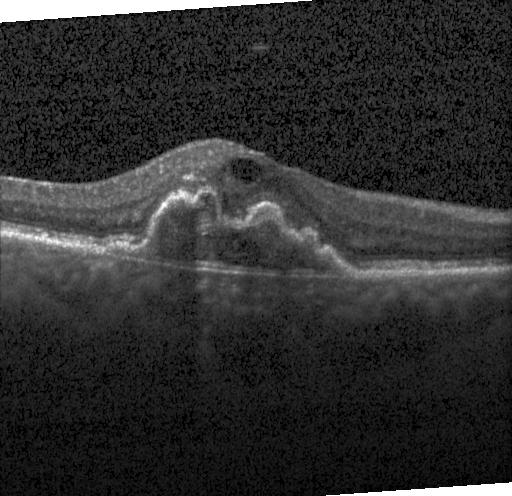 Optical coherence tomography B-scan
Diagnosis: a choroidal neovascular membrane.